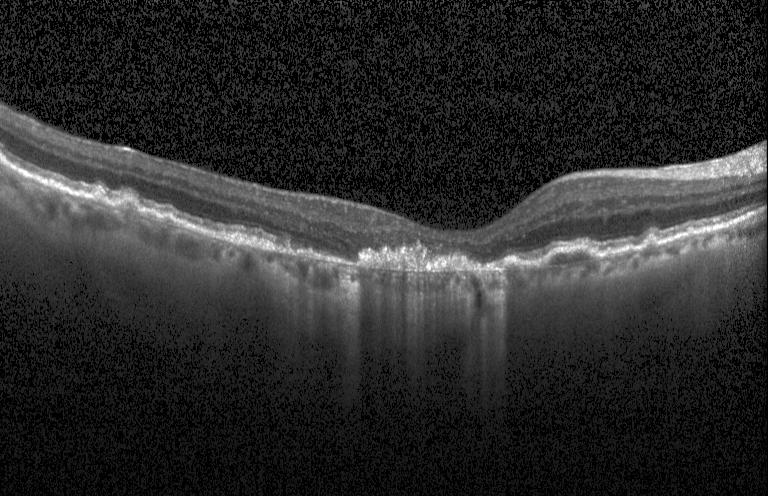

Choroidal neovascularization (CNV).